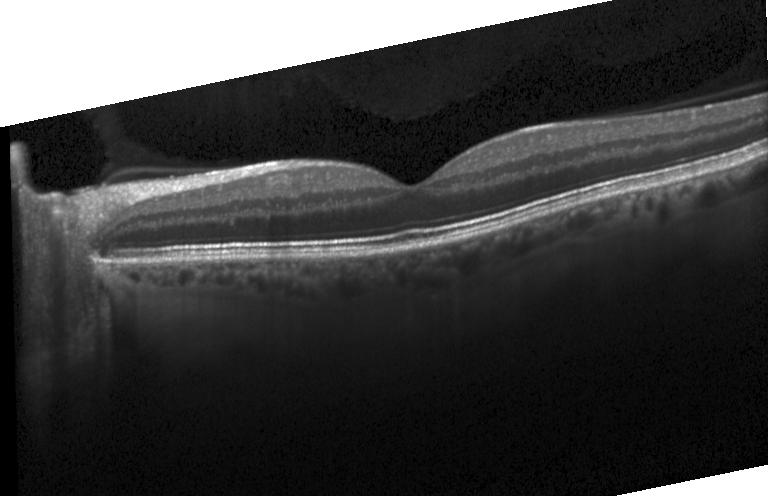
Retinal OCT cross-section, acquired on a Heidelberg Spectralis
Finding: no choroidal neovascularization, diabetic macular edema, or drusen.